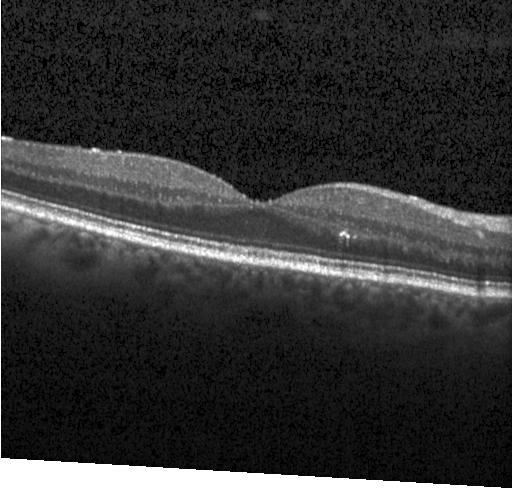
OCT scan showing no evidence of choroidal neovascularization, diabetic macular edema, or drusen.